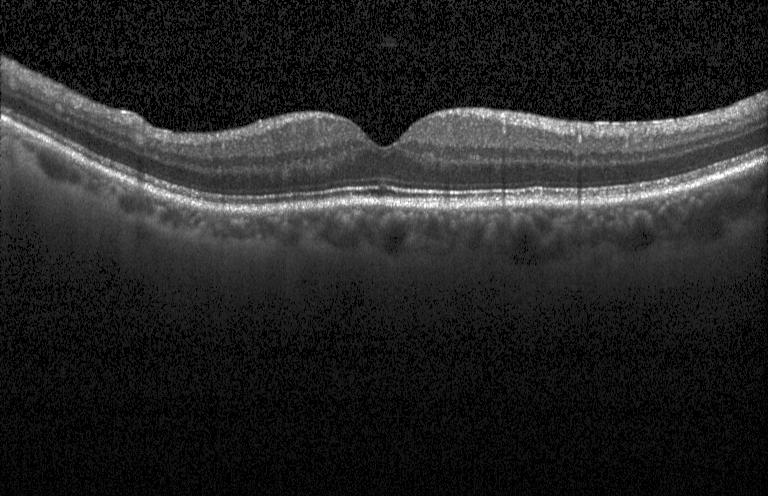 Retinal OCT B-scan; spectral-domain OCT — The scan shows no choroidal neovascularization, diabetic macular edema, or drusen.